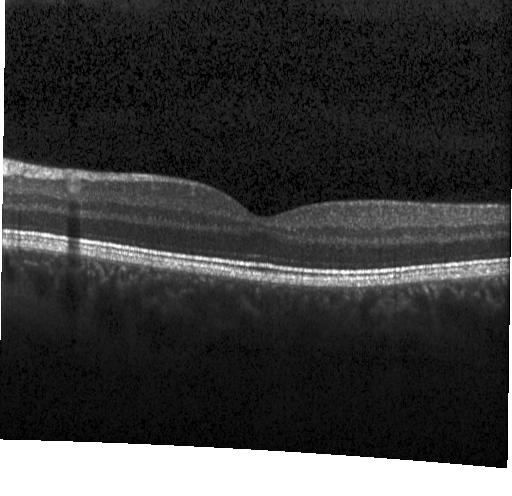

Heidelberg Spectralis. Optical coherence tomography B-scan
OCT finding: no choroidal neovascularization, no diabetic macular edema, and no drusen.